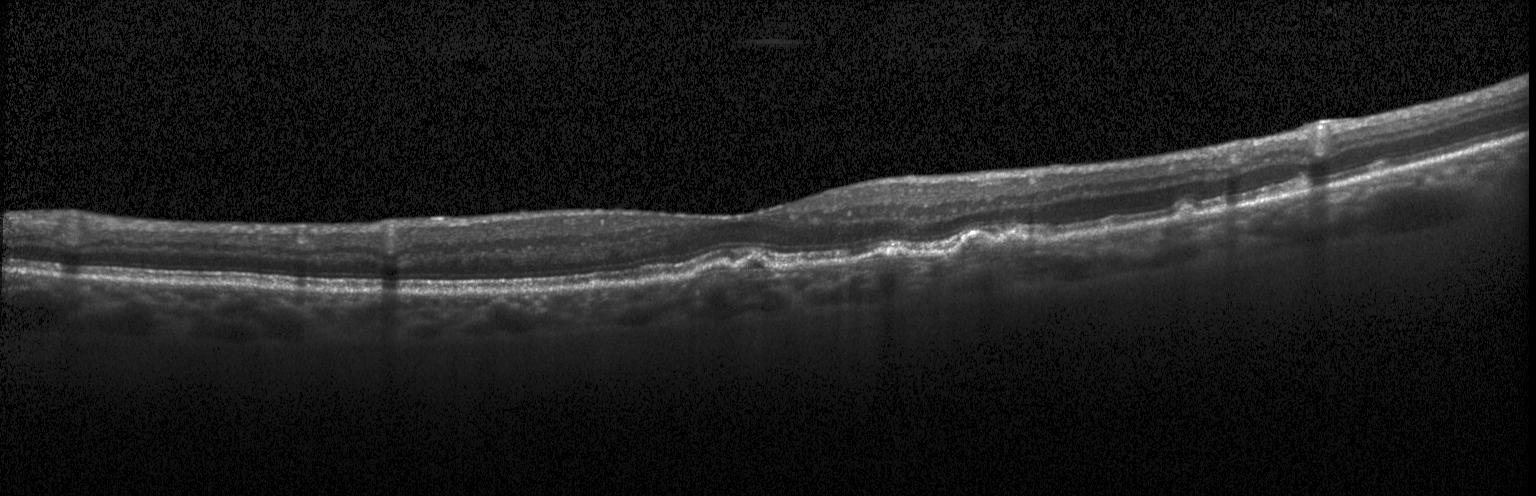

Retinal OCT B-scan
Finding: multiple drusen.